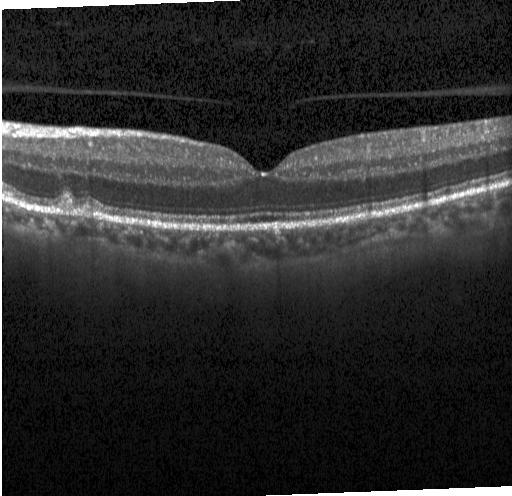

Retinal OCT B-scan.
Multiple drusen.